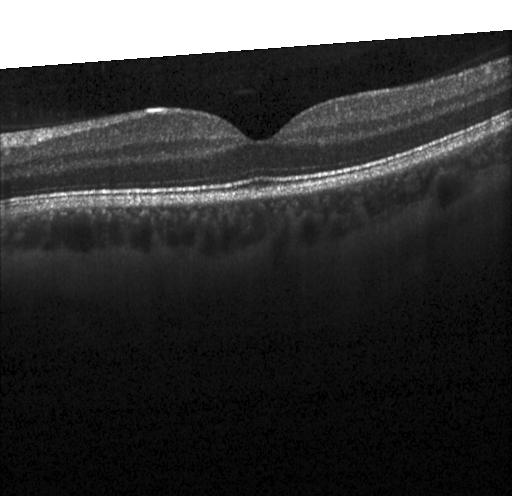

OCT B-scan, Heidelberg Spectralis OCT system, centered on the fovea
Diagnosis: no evidence of choroidal neovascularization, diabetic macular edema, or drusen.